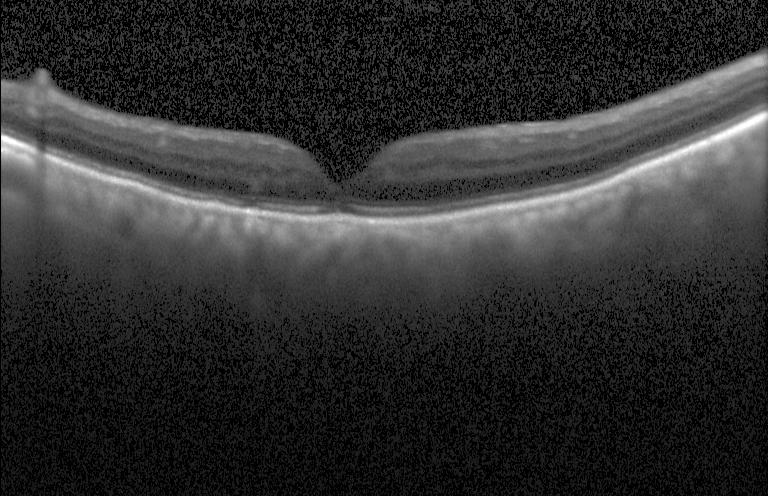
Fovea-centered, Heidelberg Spectralis, SD-OCT, OCT line scan.
Diagnosis: no CNV, no DME, and no drusen.